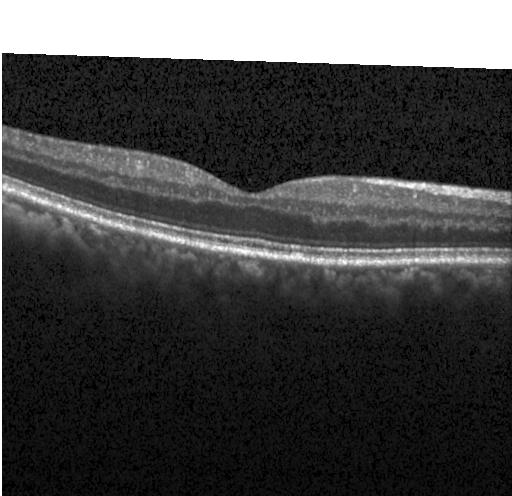 Retinal OCT B-scan — Assessment: no evidence of choroidal neovascularization, diabetic macular edema, or drusen.